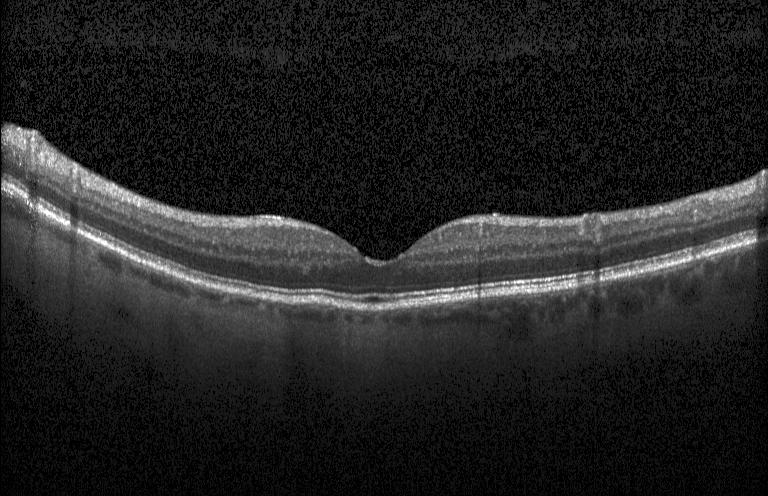
This B-scan demonstrates neither choroidal neovascularization, diabetic macular edema, nor drusen.